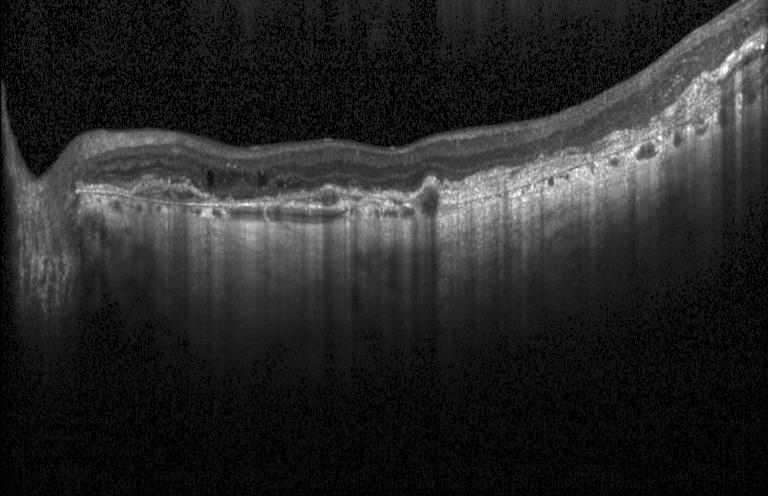
OCT scan showing a choroidal neovascular membrane.